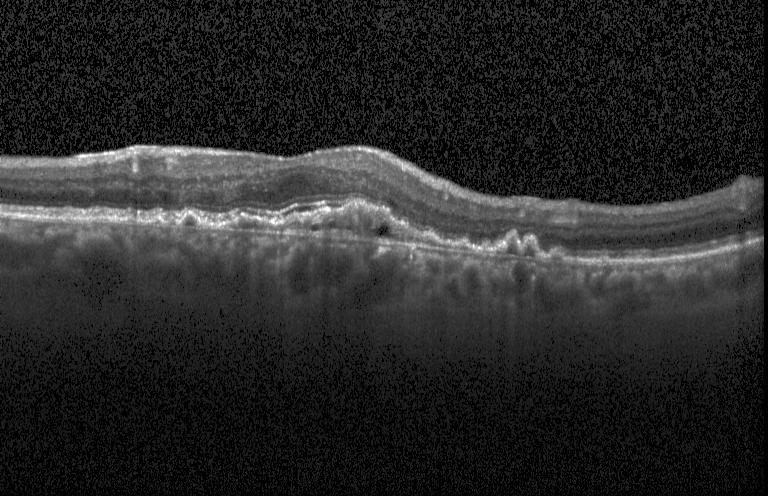
OCT scan showing a choroidal neovascular membrane.